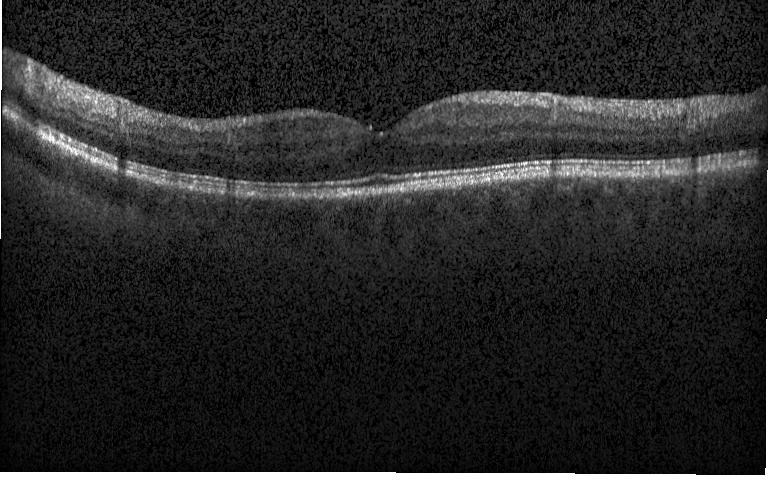
This B-scan demonstrates no CNV, DME, or drusen.